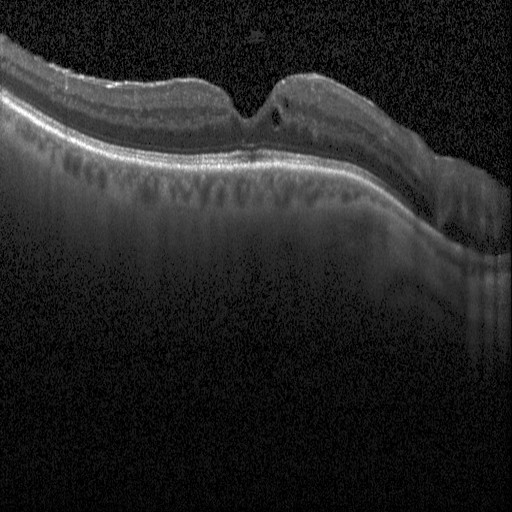
Retinal OCT B-scan.
Dx: diabetic macular edema.